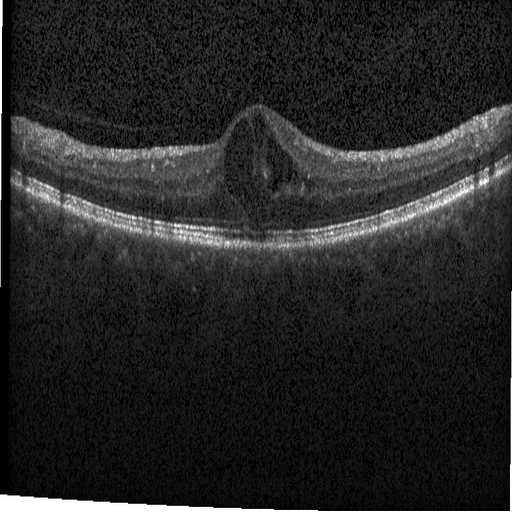
Spectral-domain OCT B-scan: diabetic macular edema (DME).